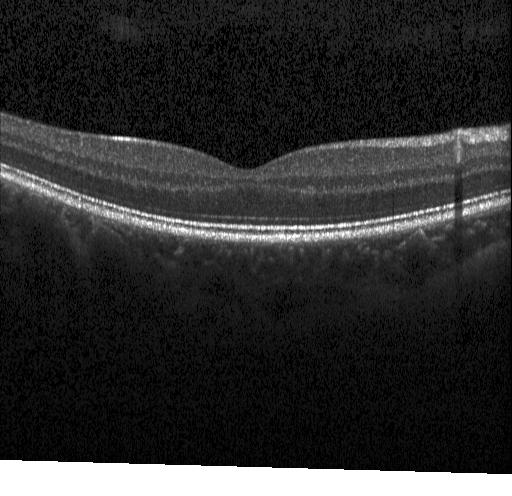

Through the macula · spectral-domain optical coherence tomography · Heidelberg Spectralis OCT system · OCT line scan — This B-scan demonstrates neither choroidal neovascularization, diabetic macular edema, nor drusen.